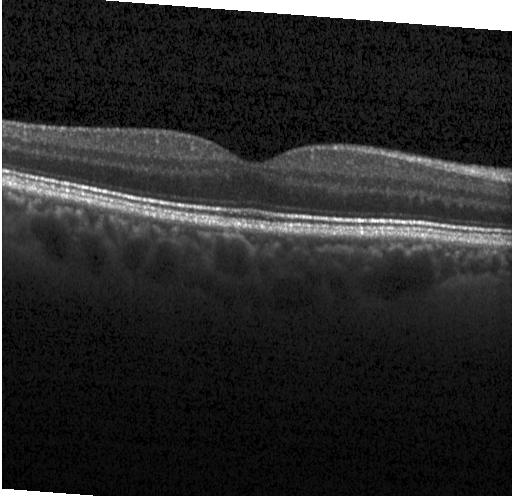 Macular scan · optical coherence tomography scan · Heidelberg Spectralis · spectral-domain OCT.
The scan shows no choroidal neovascularization, diabetic macular edema, or drusen.